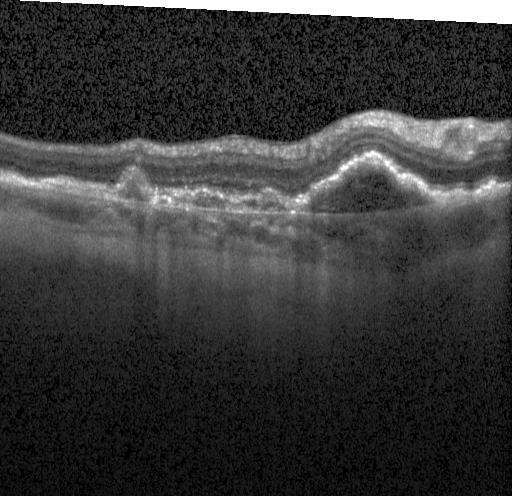
OCT scan showing a choroidal neovascular membrane.